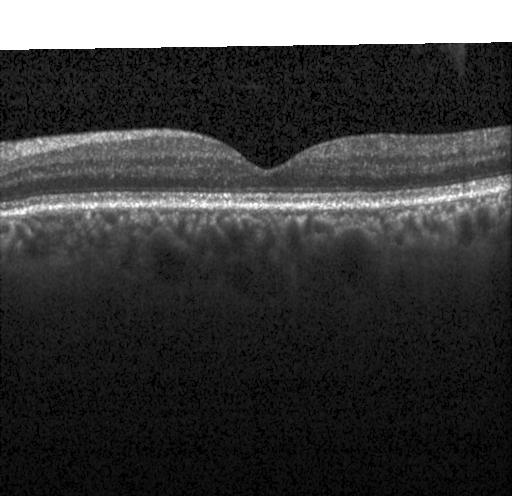 Spectral-domain OCT; Heidelberg Spectralis OCT system; retinal OCT cross-section; through the macula
Assessment: no choroidal neovascularization, no diabetic macular edema, and no drusen.